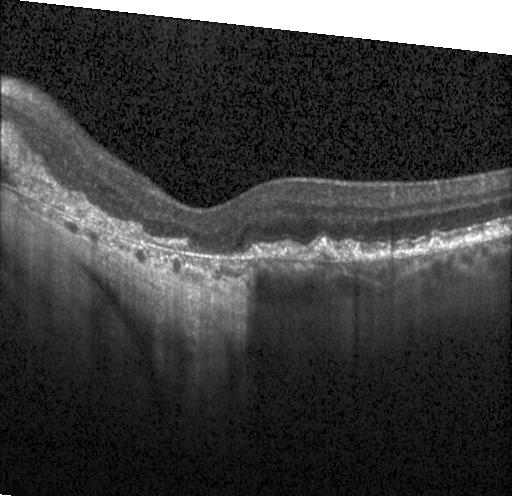
Optical coherence tomography B-scan; instrument: Heidelberg Spectralis
This B-scan demonstrates choroidal neovascularization (CNV).